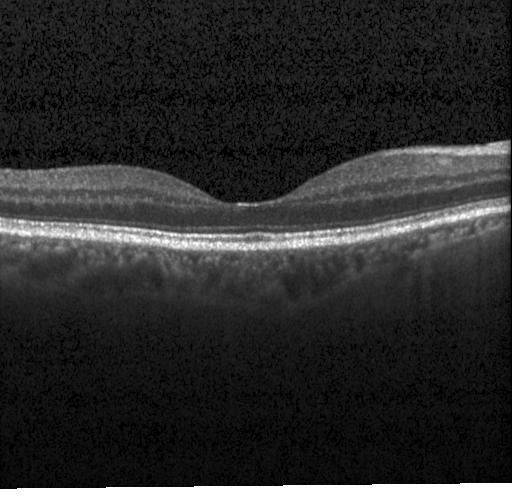
Centered on the fovea. Optical coherence tomography scan. Acquired on a Heidelberg Spectralis.
Dx: no CNV, no DME, and no drusen.